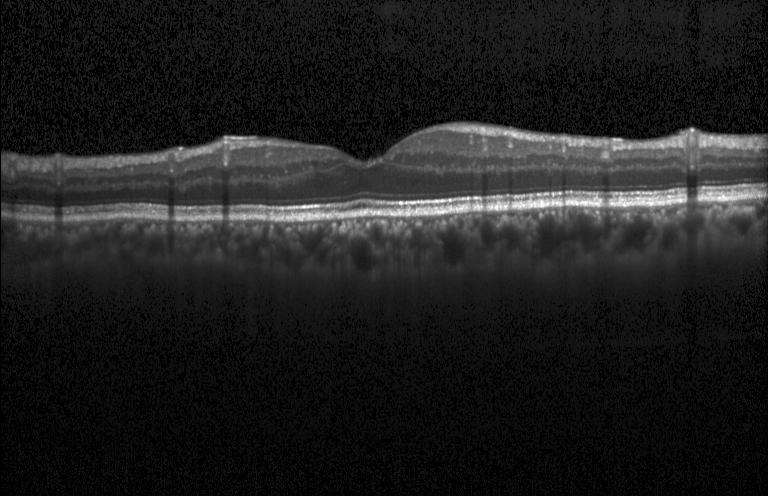
Through the macula; optical coherence tomography scan; instrument: Heidelberg Spectralis; spectral-domain OCT — Finding: no CNV, DME, or drusen.